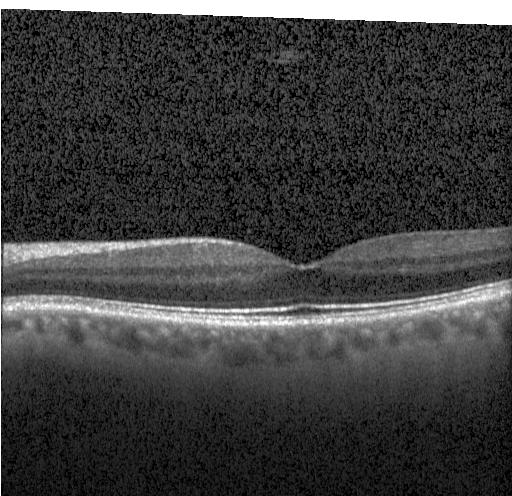

SD-OCT · optical coherence tomography scan · Heidelberg Spectralis · horizontal scan through the fovea. Finding: no choroidal neovascularization, diabetic macular edema, or drusen.